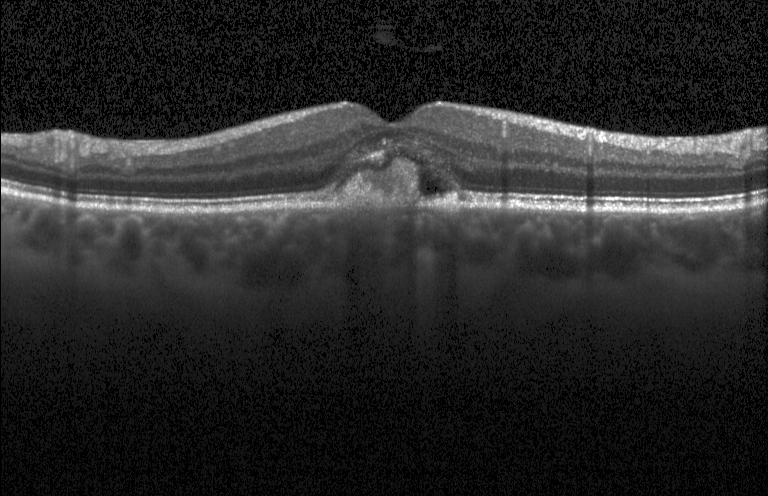

Retinal OCT cross-section · fovea-centered · spectral-domain OCT · acquired on a Heidelberg Spectralis — A choroidal neovascular membrane.